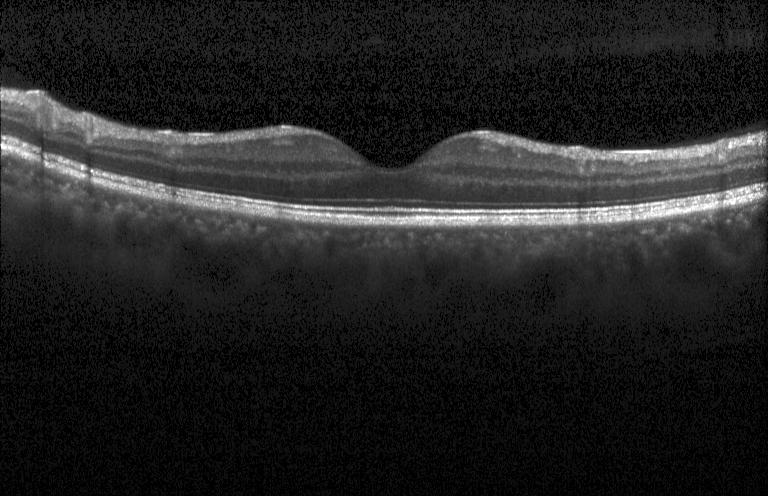 Spectral-domain OCT B-scan: no CNV, no DME, and no drusen.